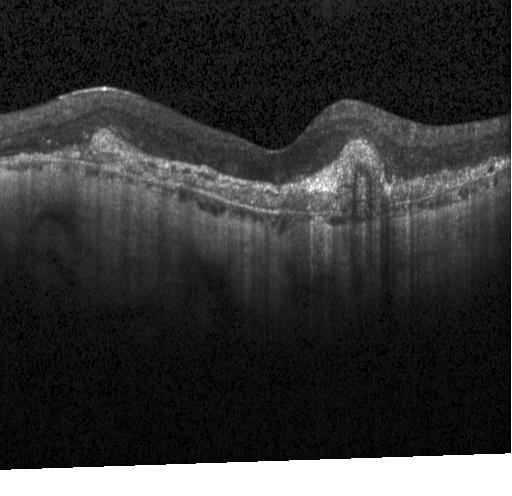

SD-OCT. Heidelberg Spectralis OCT system. Retinal OCT cross-section. Fovea-centered — Diagnosis: a choroidal neovascular membrane.